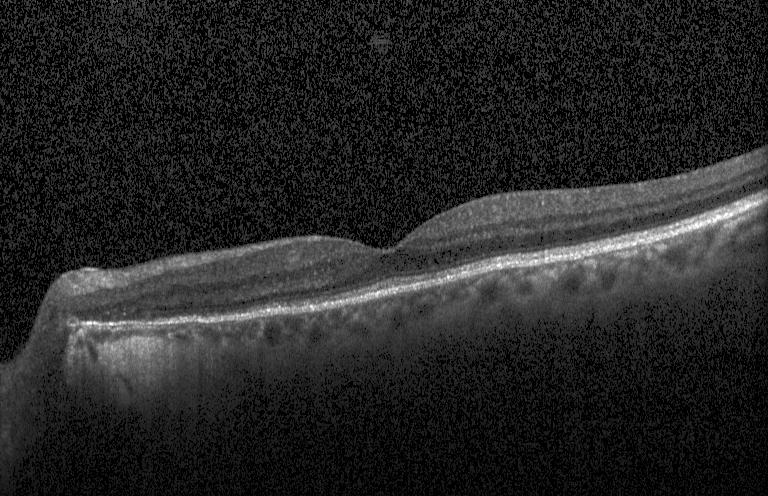 Horizontal scan through the fovea. OCT B-scan. SD-OCT. Acquired on a Heidelberg Spectralis. Assessment: no choroidal neovascularization, no diabetic macular edema, and no drusen.